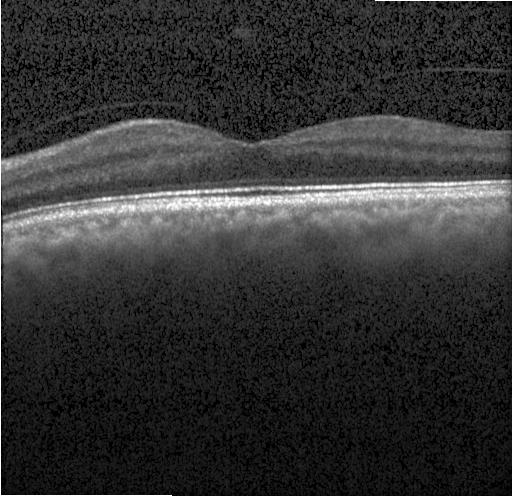

Diagnosis: no CNV, no DME, and no drusen.